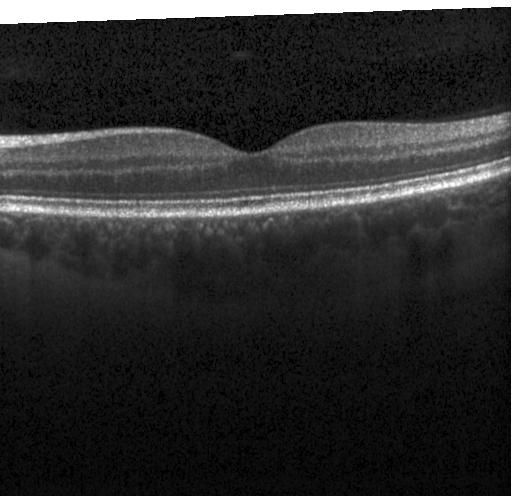 Optical coherence tomography B-scan. SD-OCT.
This B-scan demonstrates no CNV, DME, or drusen.